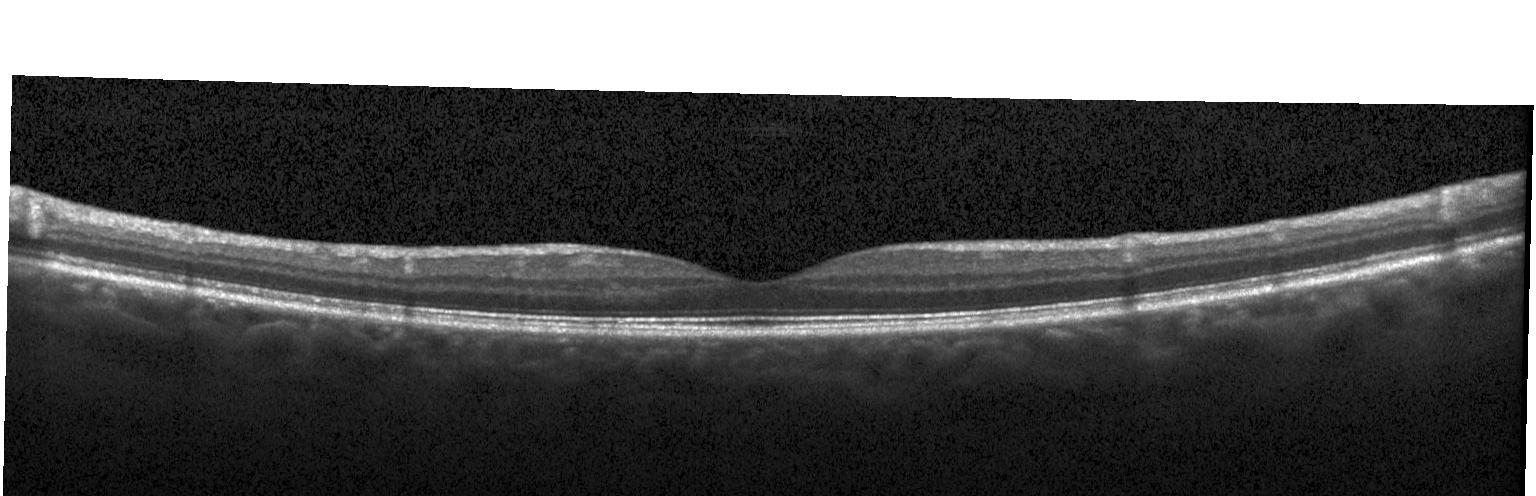

Diagnosis: no CNV, DME, or drusen.